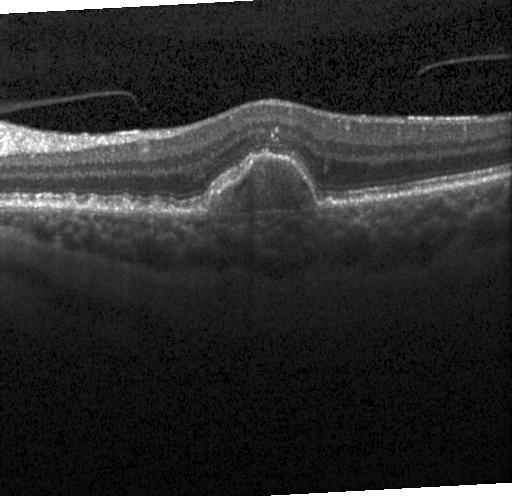

Optical coherence tomography B-scan. Choroidal neovascularization.